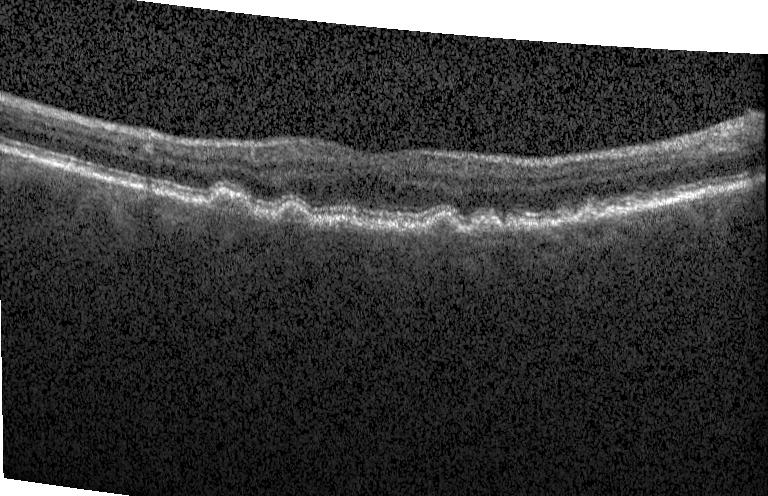
The scan shows drusen.